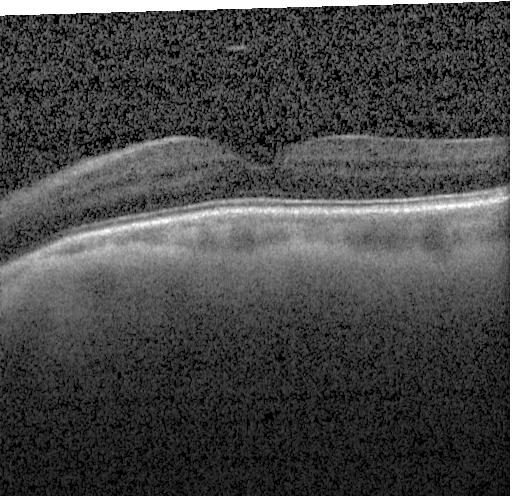

Diagnosis: neither choroidal neovascularization, diabetic macular edema, nor drusen.